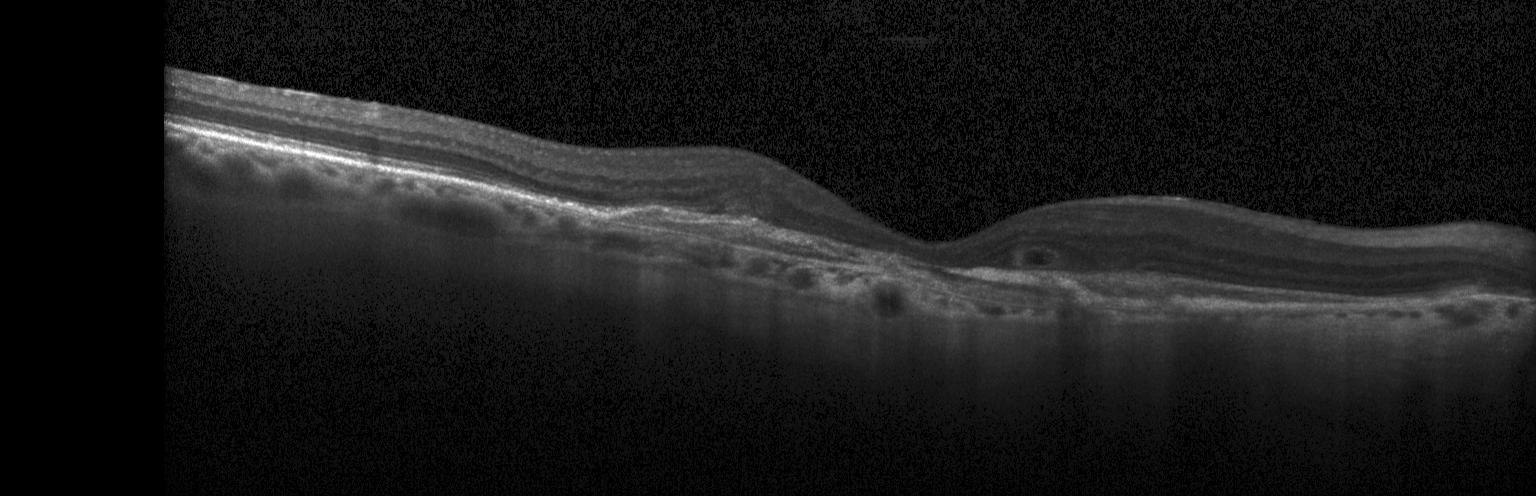
OCT B-scan, through the macula, spectral-domain OCT, instrument: Heidelberg Spectralis
Impression: CNV.